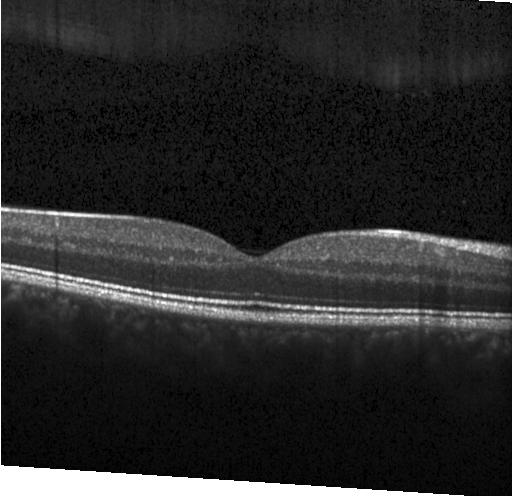 Assessment: no evidence of CNV, DME, or drusen.